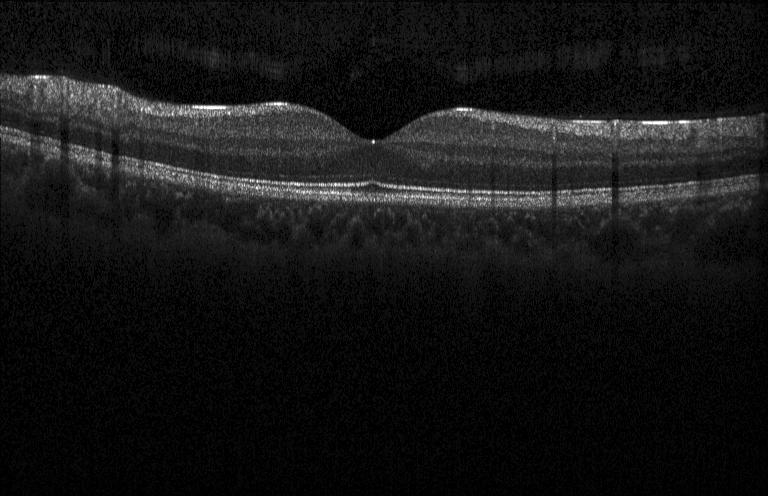

Finding: neither choroidal neovascularization, diabetic macular edema, nor drusen.